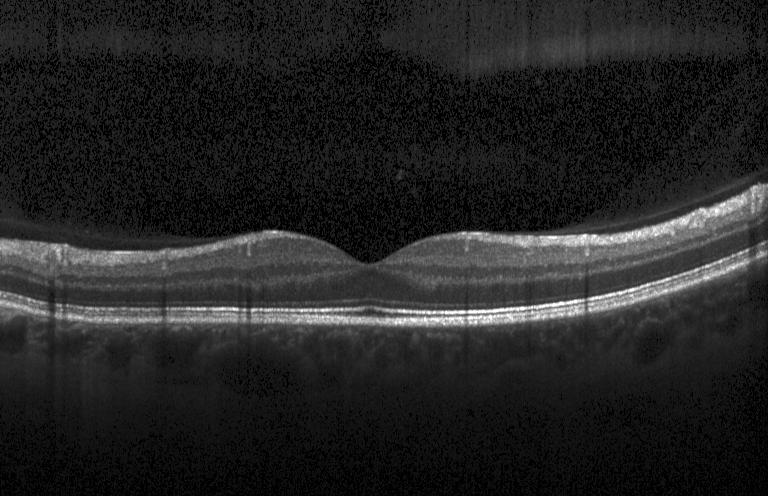

Diagnosis: neither CNV, DME, nor drusen.